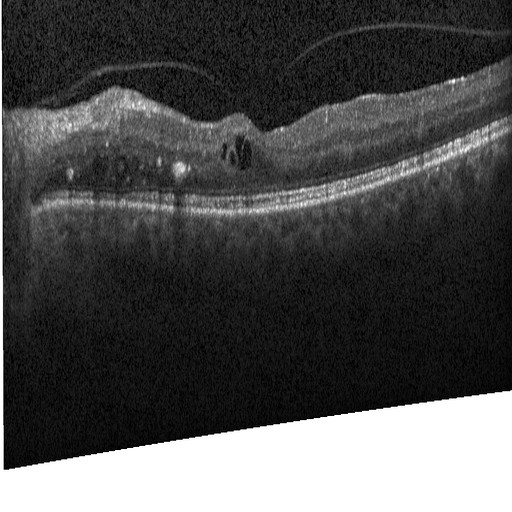
Heidelberg Spectralis OCT system; retinal OCT cross-section; through the macula — Dx: diabetic macular edema.